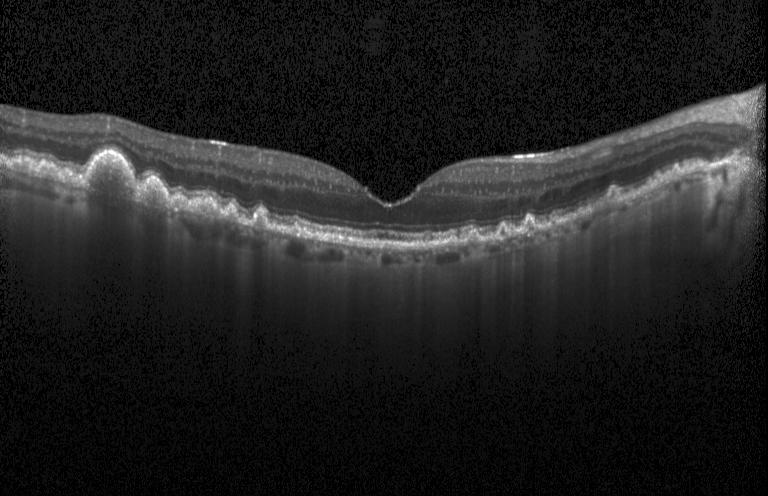 Fovea-centered, spectral-domain optical coherence tomography, instrument: Heidelberg Spectralis, retinal OCT B-scan.
The scan shows sub-RPE drusenoid deposits.